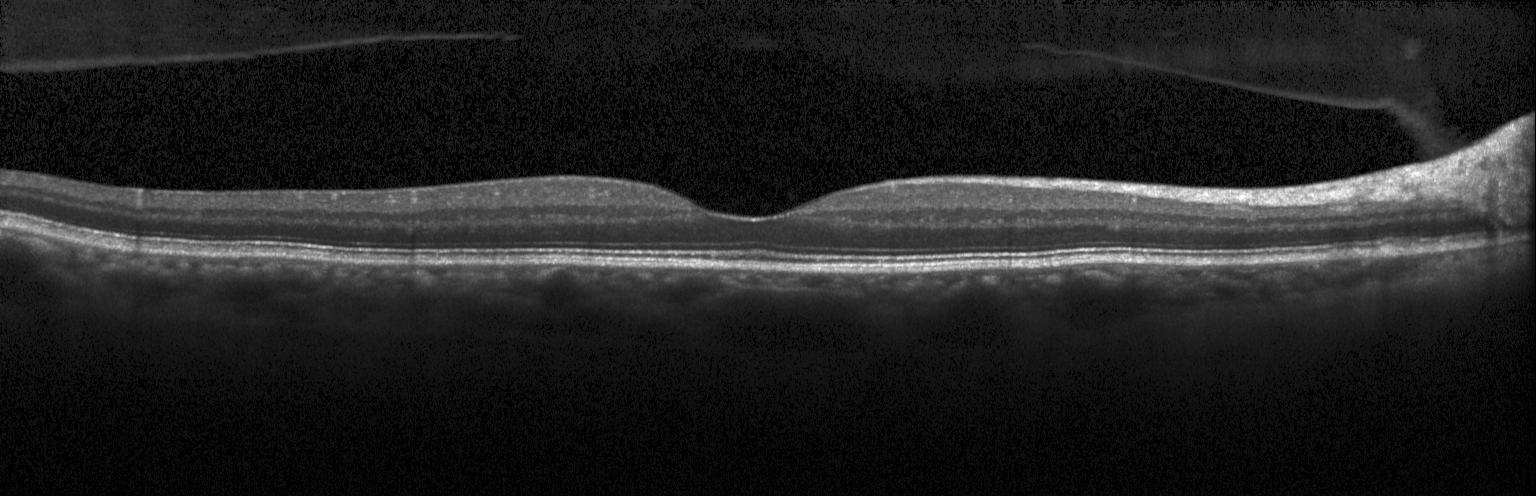

Instrument: Heidelberg Spectralis; horizontal scan through the fovea; retinal OCT B-scan — Diagnosis: neither choroidal neovascularization, diabetic macular edema, nor drusen.